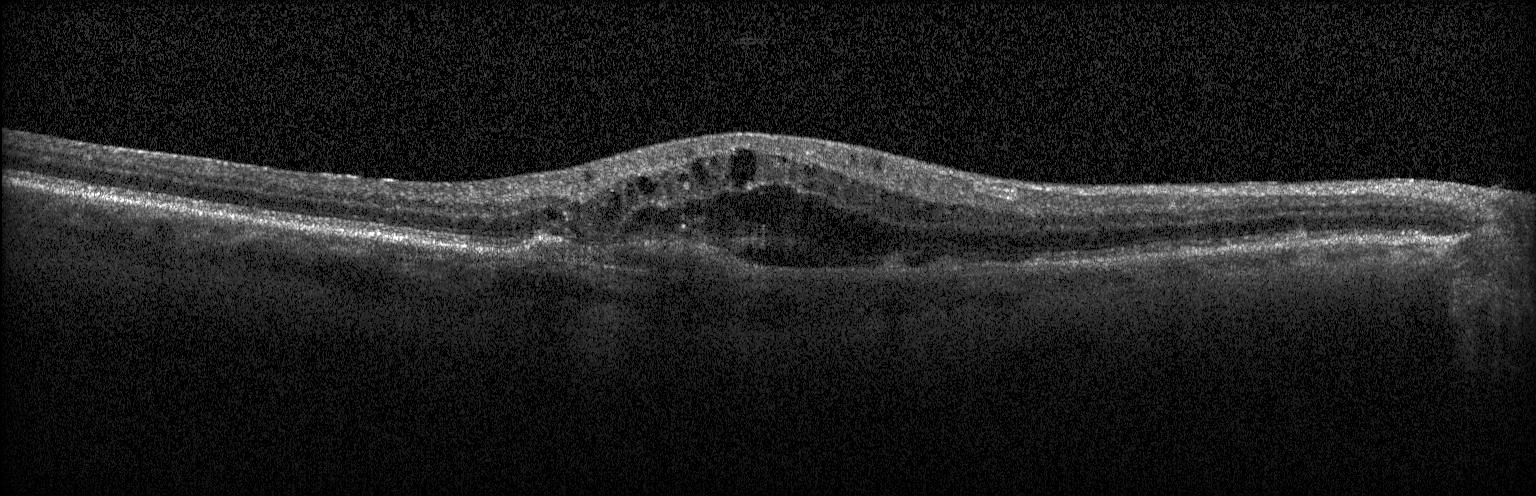

Impression: a choroidal neovascular membrane.